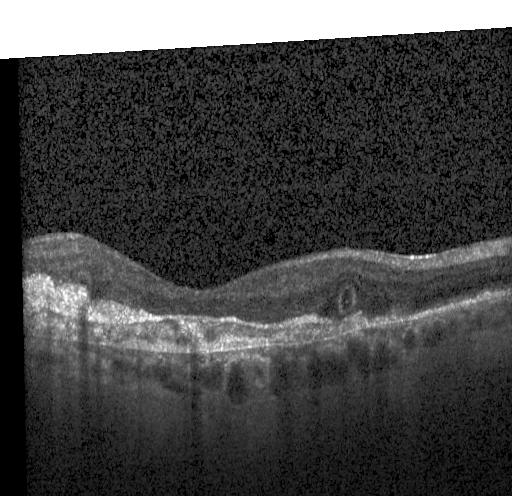
Instrument: Heidelberg Spectralis, retinal OCT B-scan, spectral-domain OCT
Diagnosis: CNV.